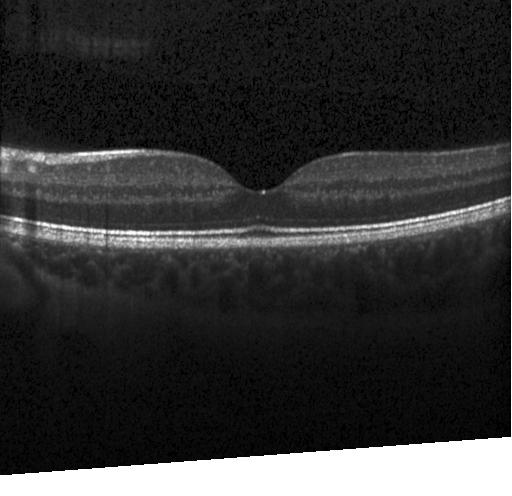 OCT finding: no evidence of choroidal neovascularization, diabetic macular edema, or drusen.